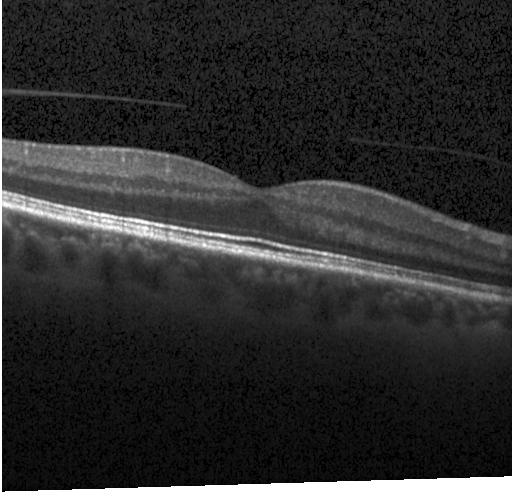
Finding: no CNV, no DME, and no drusen.